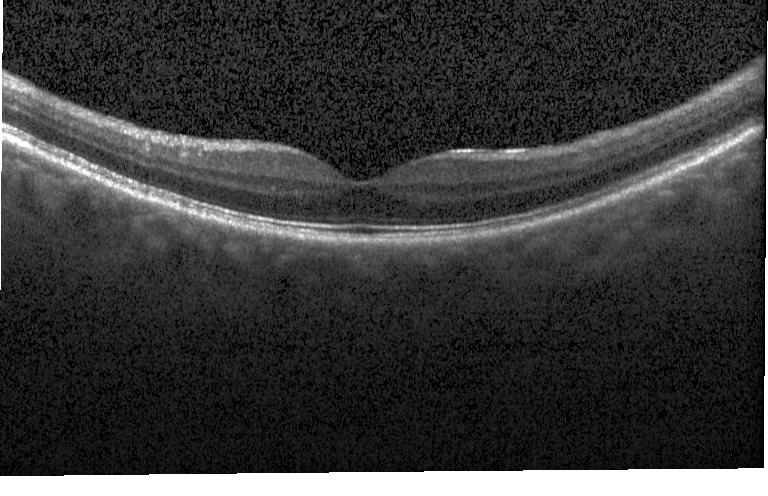

Spectral-domain OCT B-scan: no choroidal neovascularization, no diabetic macular edema, and no drusen.